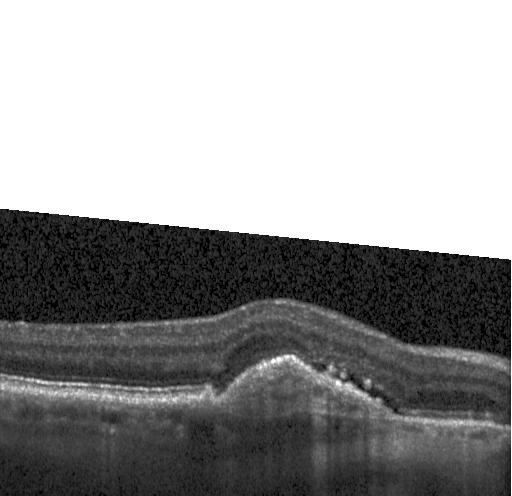 OCT scan showing choroidal neovascularization (CNV).